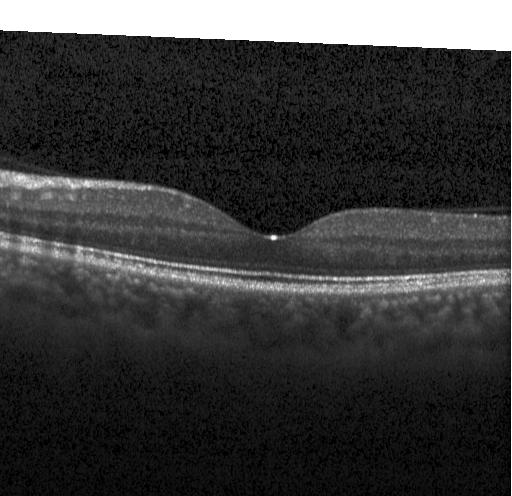
OCT B-scan. Fovea-centered. Spectral-domain optical coherence tomography.
Dx: neither choroidal neovascularization, diabetic macular edema, nor drusen.